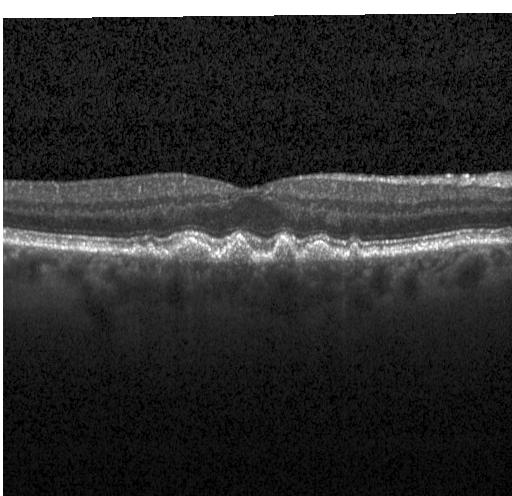

Retinal OCT B-scan. Spectral-domain optical coherence tomography
Impression: drusen.